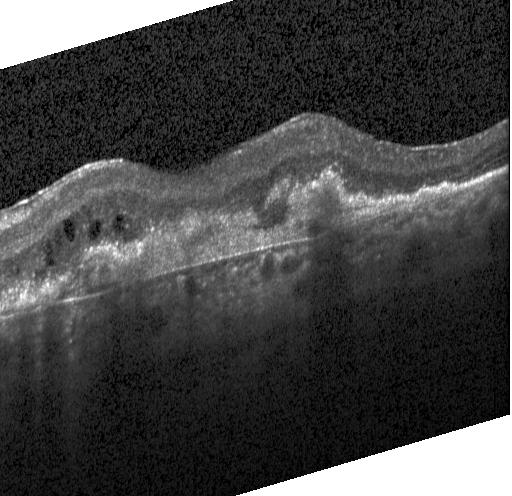 This B-scan demonstrates CNV.